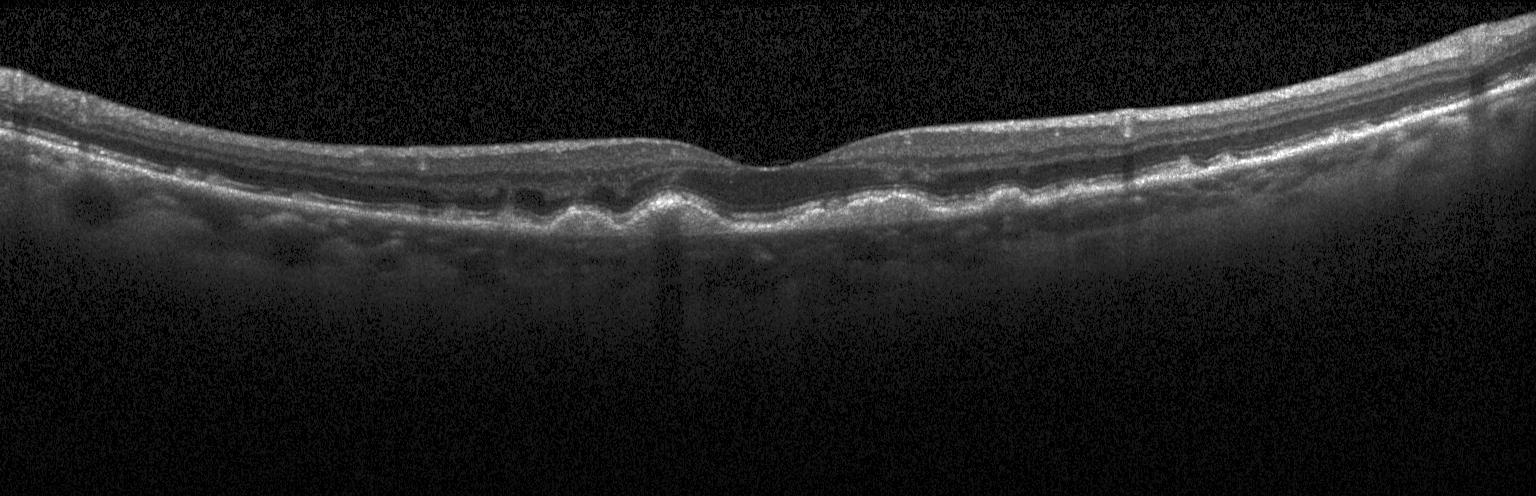

Finding: multiple drusen.